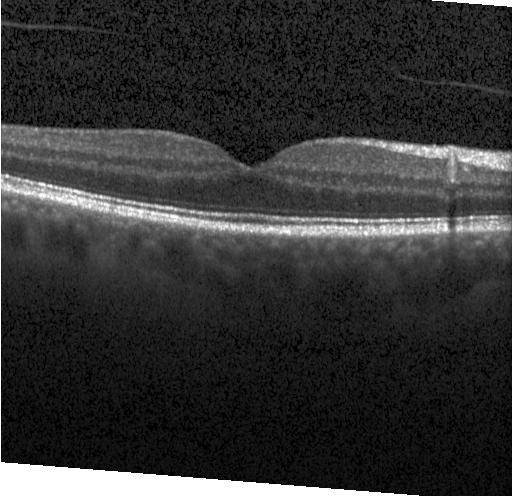

Finding: neither choroidal neovascularization, diabetic macular edema, nor drusen.